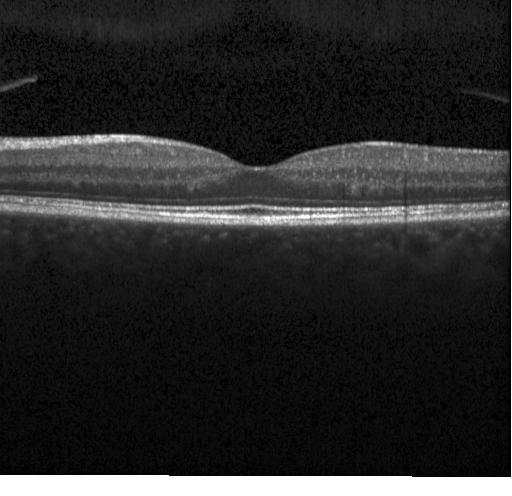
Acquired on a Heidelberg Spectralis, optical coherence tomography B-scan
Diagnosis: no evidence of CNV, DME, or drusen.